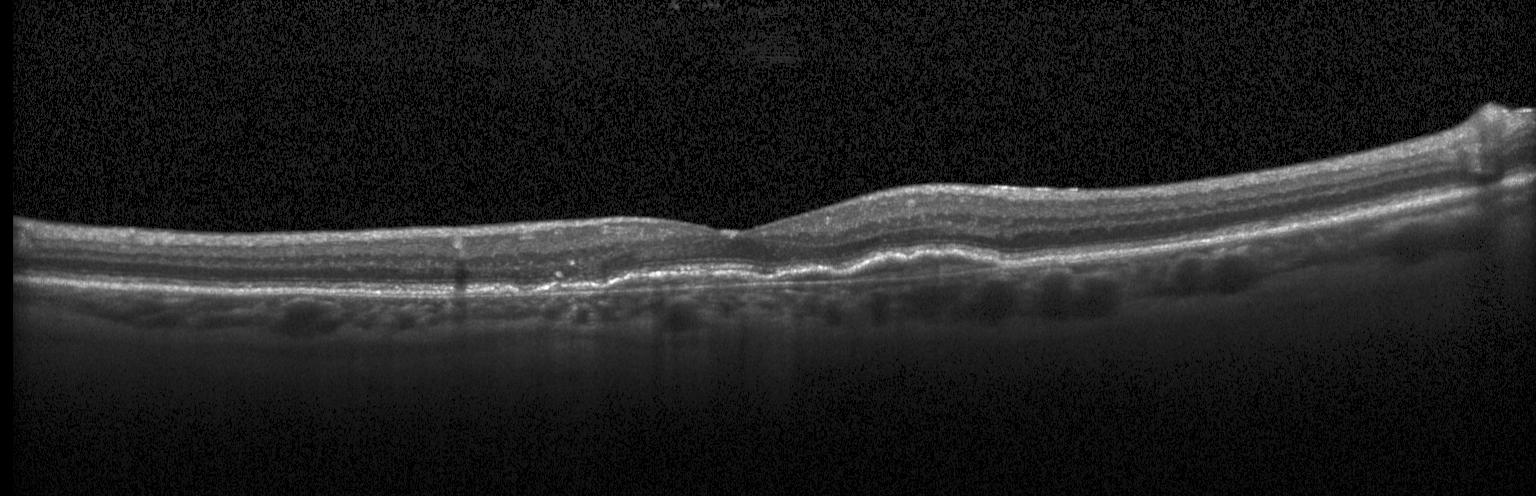

Fovea-centered. Spectral-domain OCT. Optical coherence tomography scan.
Choroidal neovascularization.